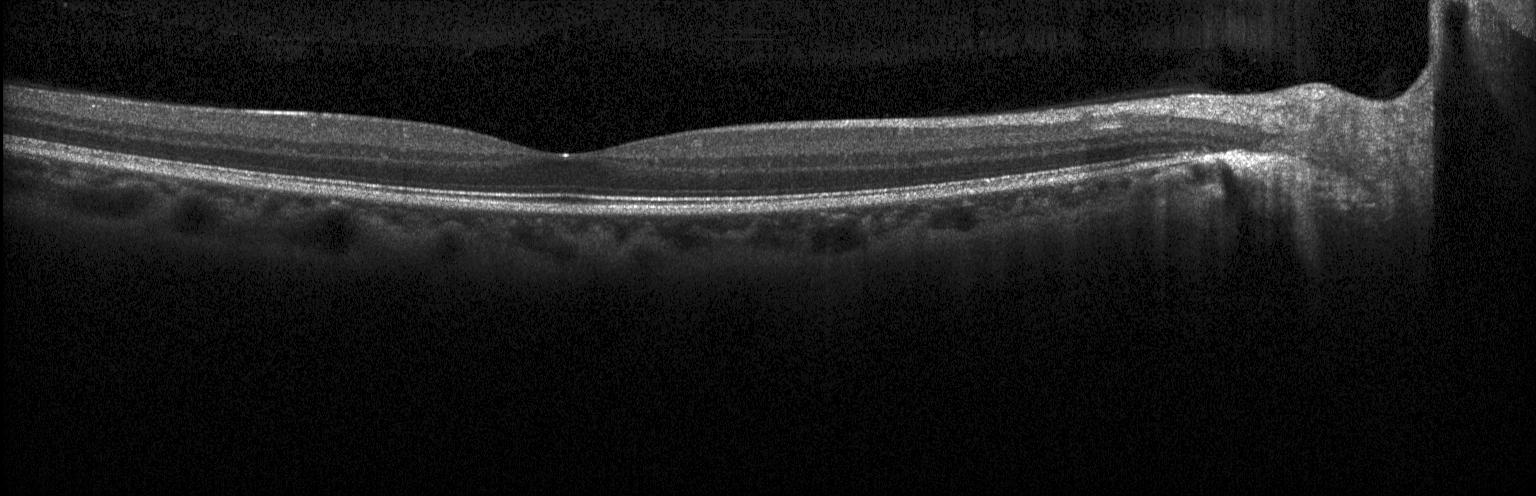

Optical coherence tomography B-scan
Diagnosis: no evidence of choroidal neovascularization, diabetic macular edema, or drusen.